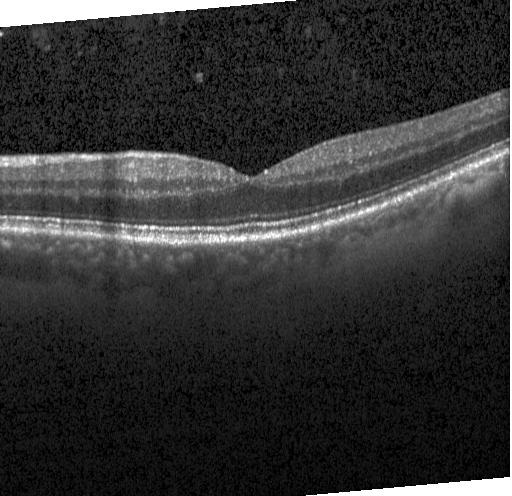 OCT line scan. Heidelberg Spectralis OCT system. SD-OCT. Macular scan — Finding: no CNV, DME, or drusen.